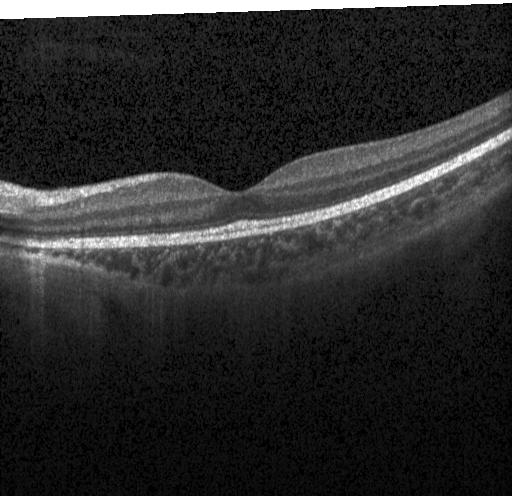

Optical coherence tomography scan — Finding: neither CNV, DME, nor drusen.